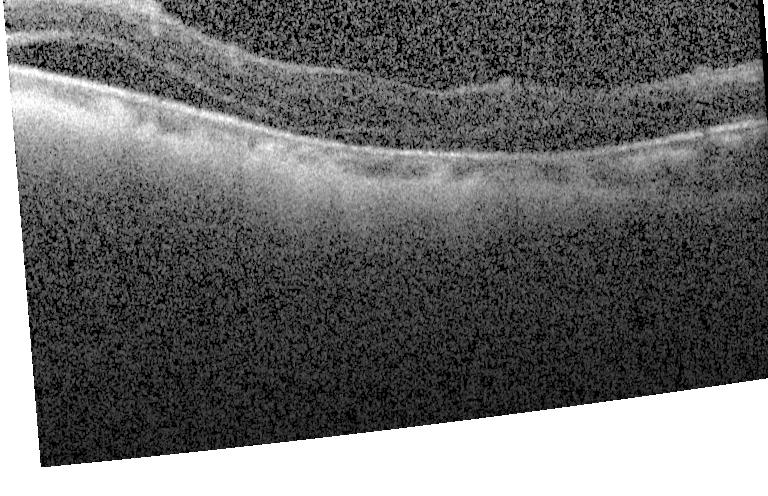 Impression: choroidal neovascularization.